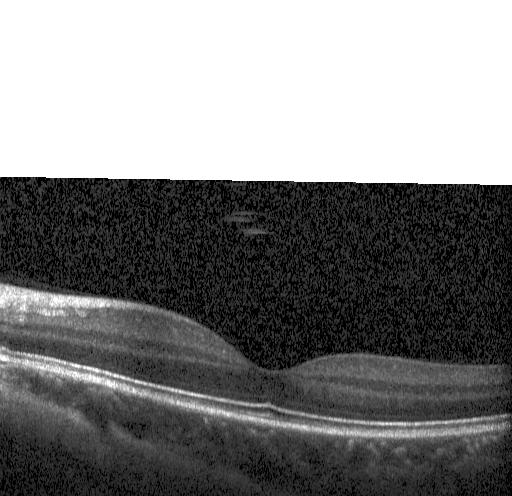 Optical coherence tomography scan.
Finding: no choroidal neovascularization, no diabetic macular edema, and no drusen.